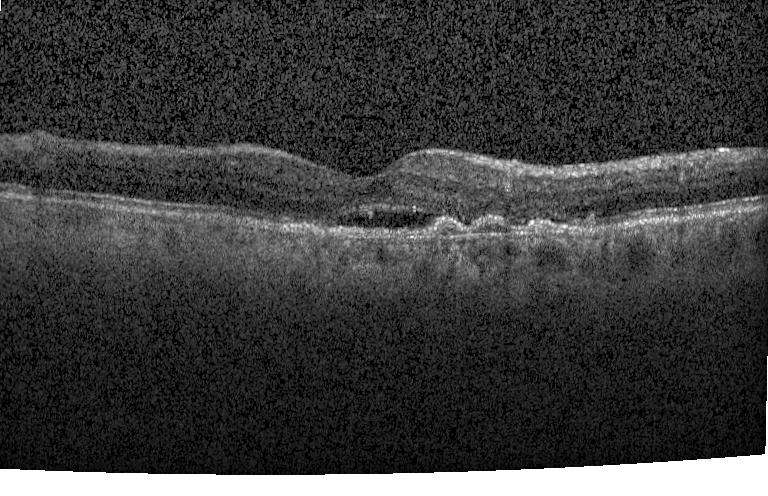
OCT scan showing choroidal neovascularization.